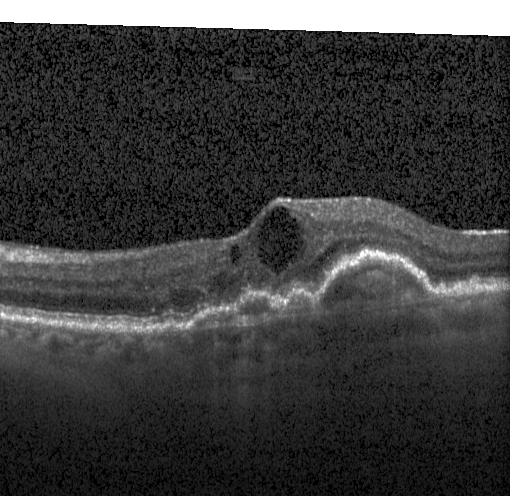
Heidelberg Spectralis, retinal OCT cross-section.
This B-scan demonstrates a choroidal neovascular membrane.